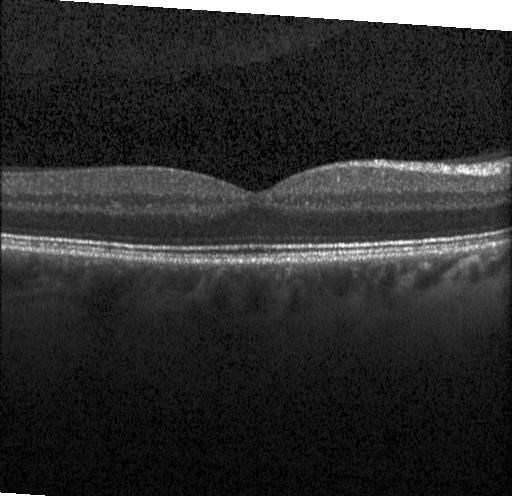

SD-OCT; OCT line scan; through the macula. Finding: neither choroidal neovascularization, diabetic macular edema, nor drusen.